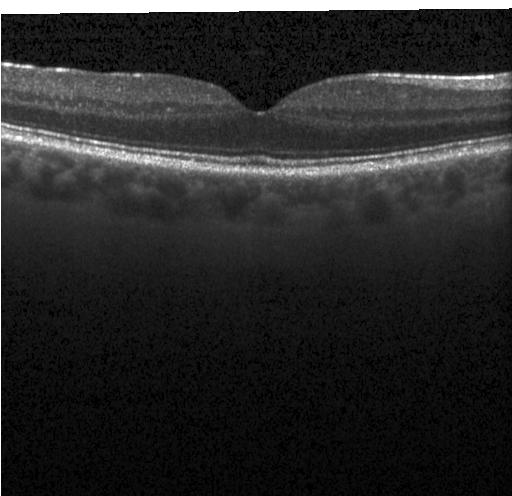

OCT finding: no choroidal neovascularization, diabetic macular edema, or drusen.